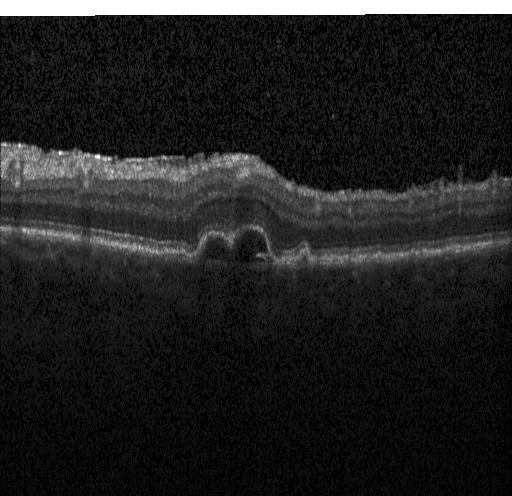
Optical coherence tomography scan
Diagnosis: choroidal neovascularization.